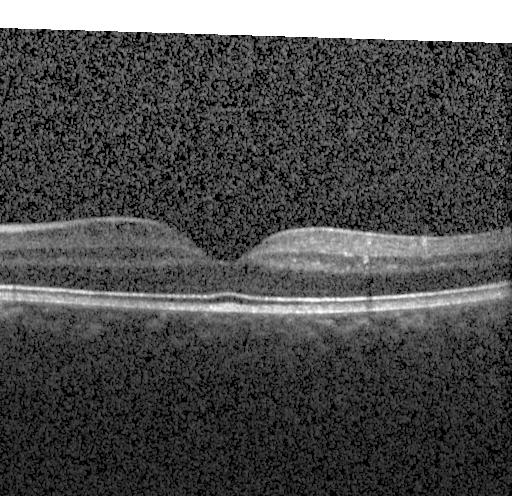
SD-OCT. OCT line scan. Through the macula. Heidelberg Spectralis.
Impression: no evidence of CNV, DME, or drusen.